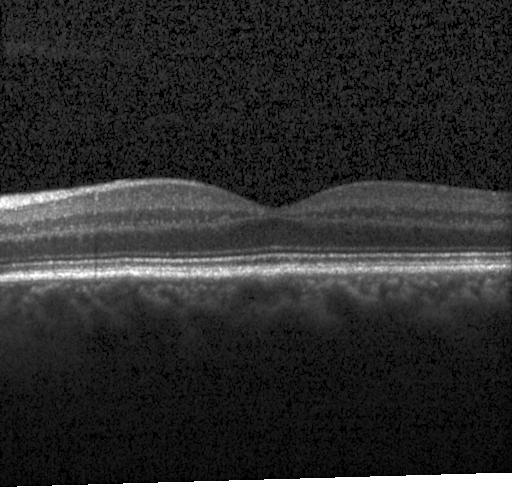
Diagnosis: no choroidal neovascularization, no diabetic macular edema, and no drusen.